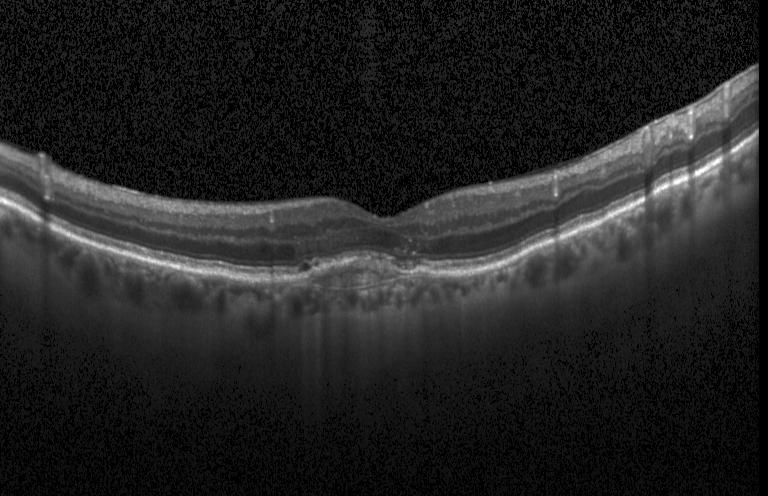

Retinal OCT B-scan
Impression: a choroidal neovascular membrane.